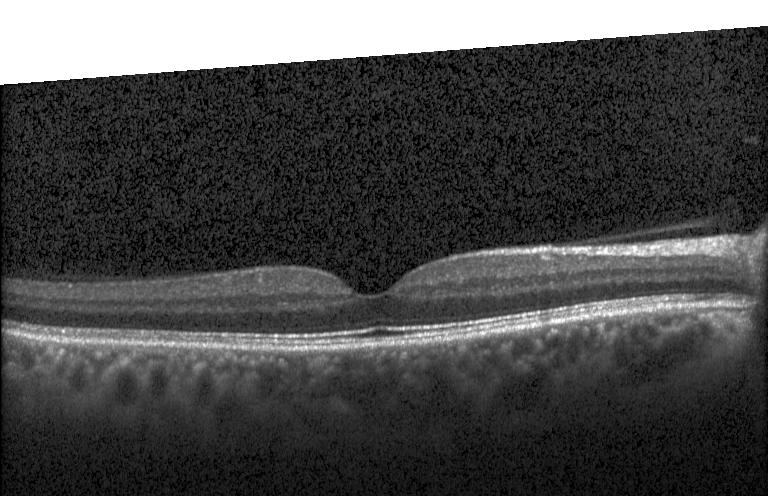
Optical coherence tomography B-scan; centered on the fovea. Impression: no choroidal neovascularization, no diabetic macular edema, and no drusen.